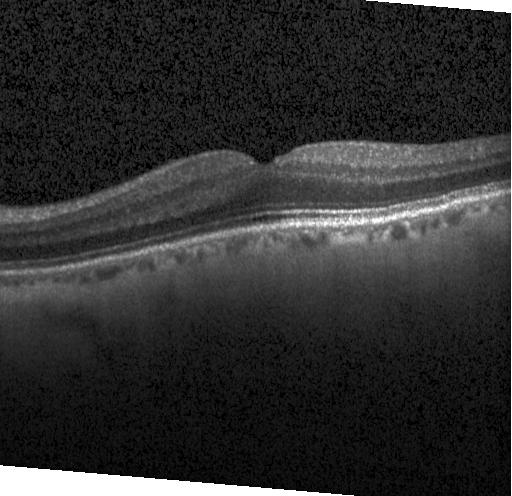 Optical coherence tomography B-scan — Diagnosis: no choroidal neovascularization, diabetic macular edema, or drusen.